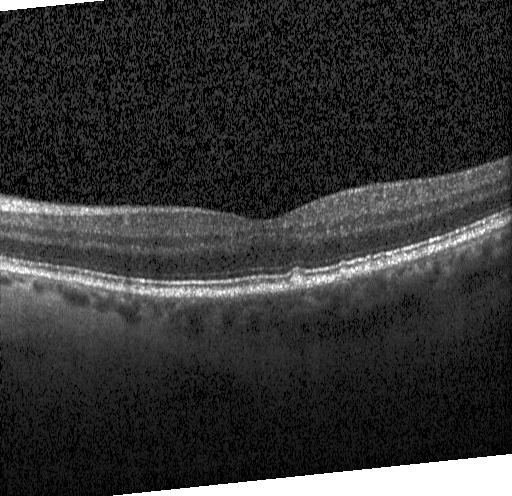

Horizontal scan through the fovea · spectral-domain optical coherence tomography · retinal OCT B-scan — This B-scan demonstrates drusen.